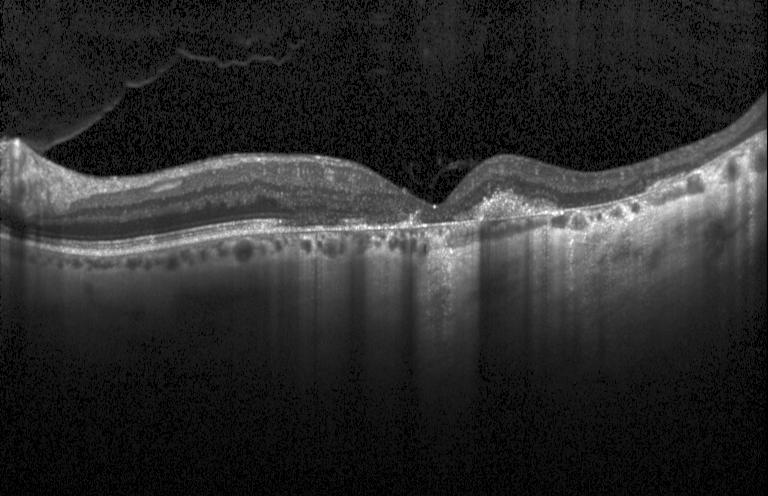 CNV.